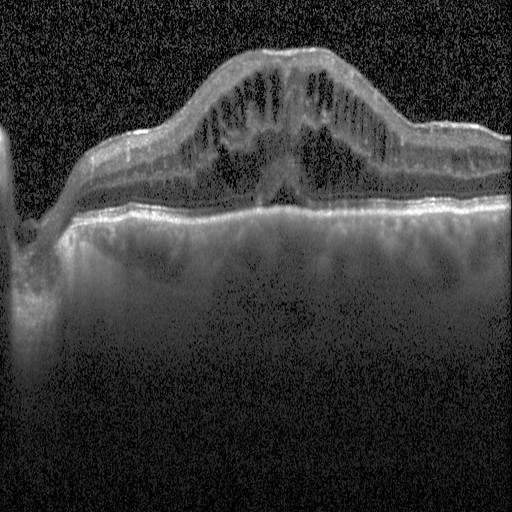 OCT B-scan.
Finding: diabetic macular edema.